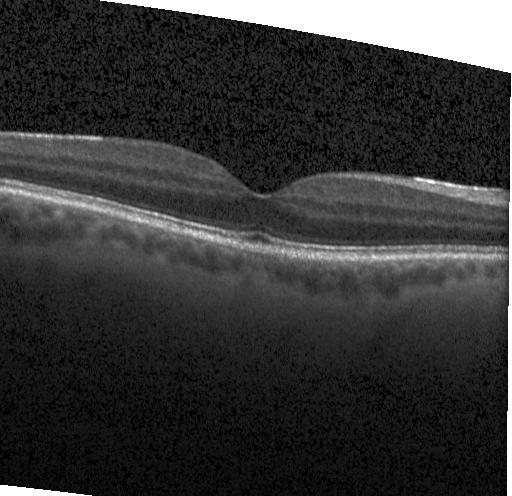 Spectral-domain OCT B-scan: no CNV, DME, or drusen.